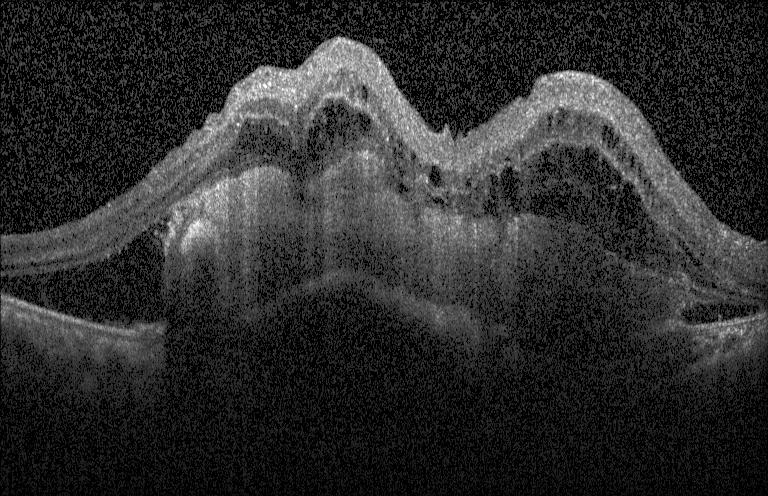

OCT B-scan
Diagnosis: a choroidal neovascular membrane.